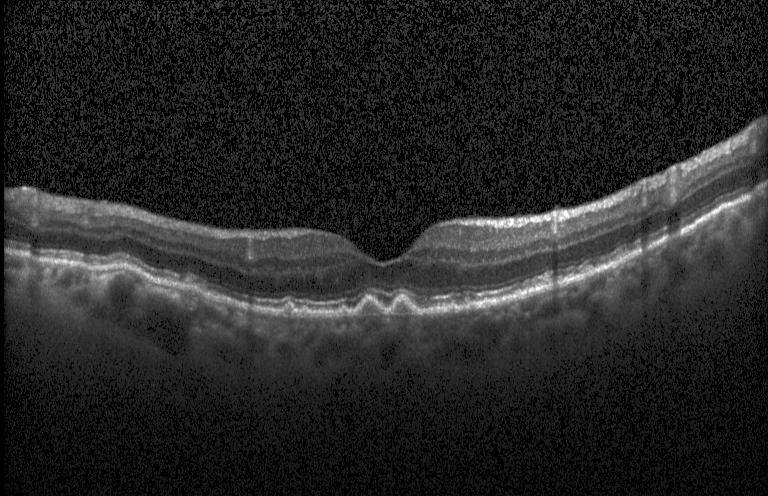

Heidelberg Spectralis OCT system, spectral-domain OCT, horizontal scan through the fovea, retinal OCT cross-section — Finding: drusen.